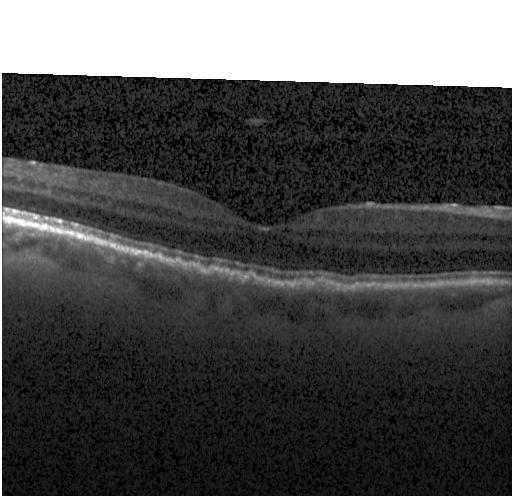 Optical coherence tomography B-scan
The scan shows sub-RPE drusenoid deposits.